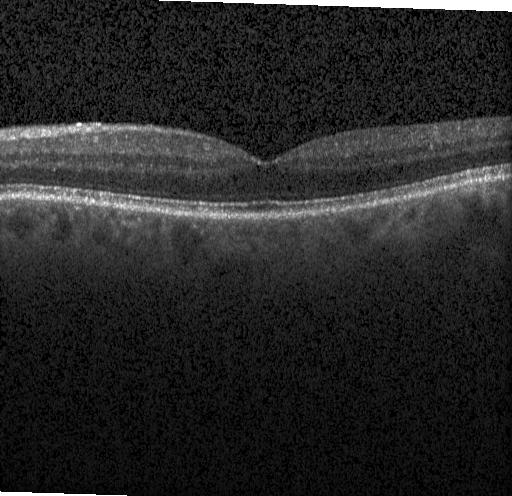

OCT line scan.
The scan shows no choroidal neovascularization, no diabetic macular edema, and no drusen.